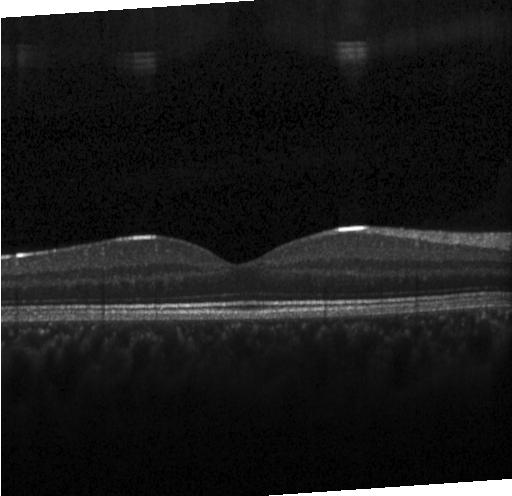

Retinal OCT cross-section showing no choroidal neovascularization, no diabetic macular edema, and no drusen.